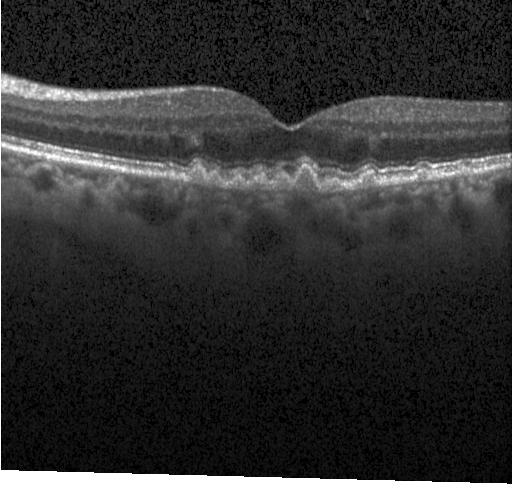 Optical coherence tomography scan · centered on the fovea · SD-OCT.
This B-scan demonstrates sub-RPE drusenoid deposits.